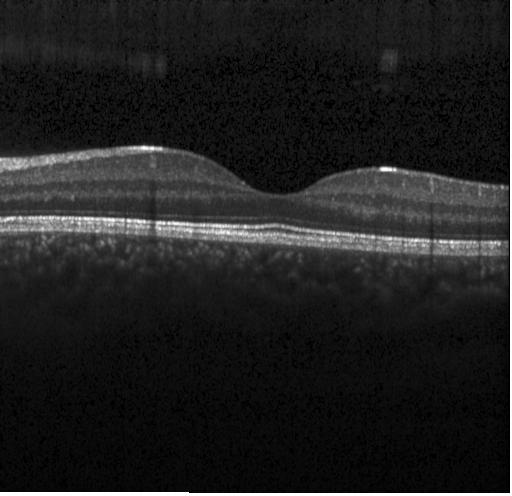
This B-scan demonstrates neither CNV, DME, nor drusen.